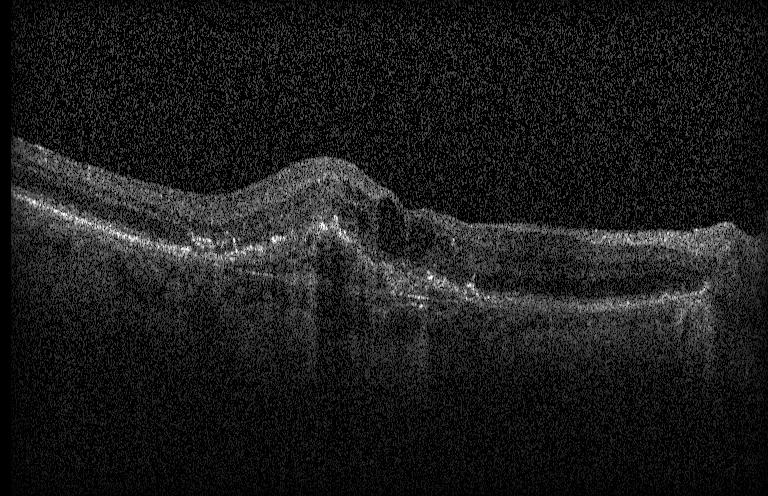

Optical coherence tomography B-scan · instrument: Heidelberg Spectralis · spectral-domain optical coherence tomography
Impression: CNV.